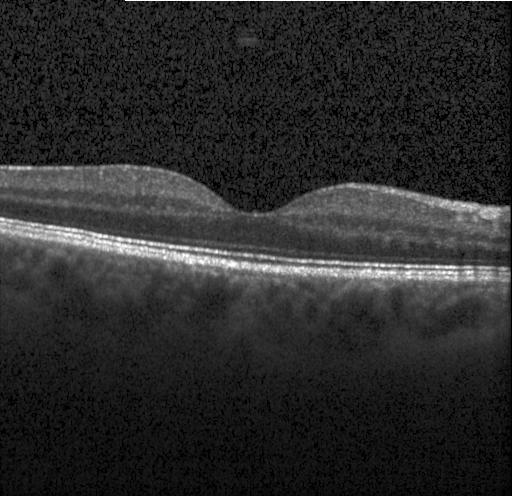

Macular scan; optical coherence tomography scan; acquired on a Heidelberg Spectralis; spectral-domain optical coherence tomography.
The scan shows no choroidal neovascularization, no diabetic macular edema, and no drusen.